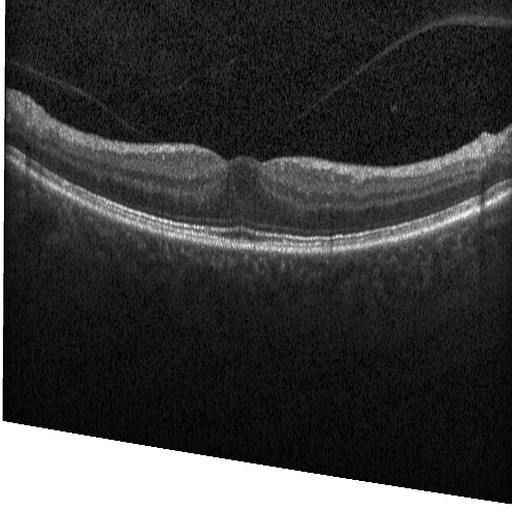

Retinal OCT B-scan
The scan shows diabetic macular edema.